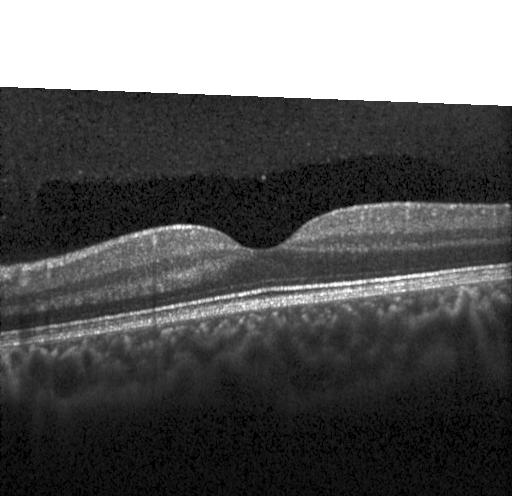
OCT B-scan showing no CNV, no DME, and no drusen.